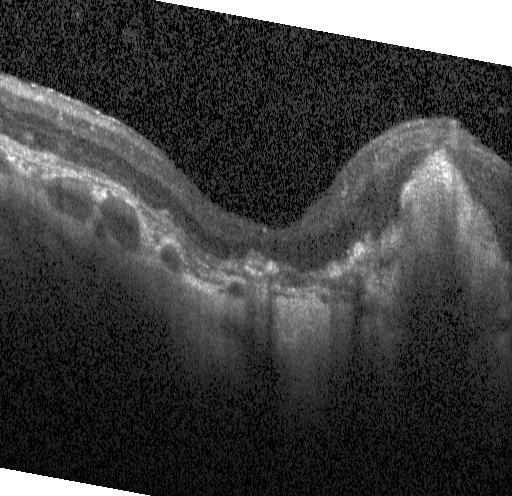 OCT B-scan. The scan shows a choroidal neovascular membrane.